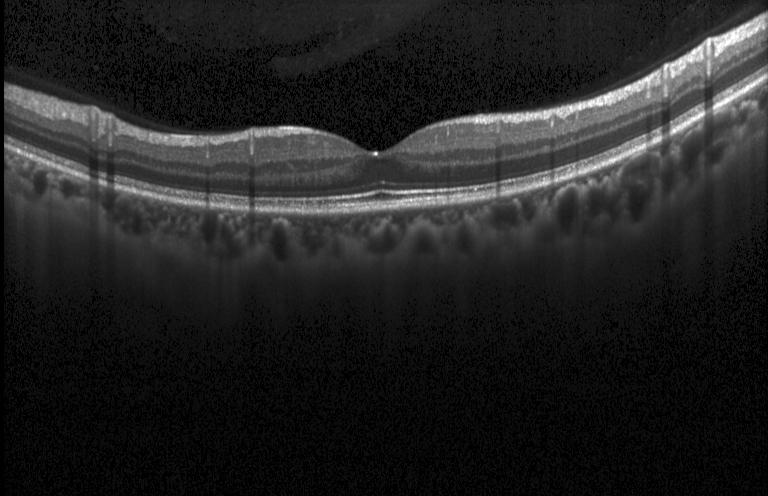 Optical coherence tomography scan.
Impression: neither CNV, DME, nor drusen.